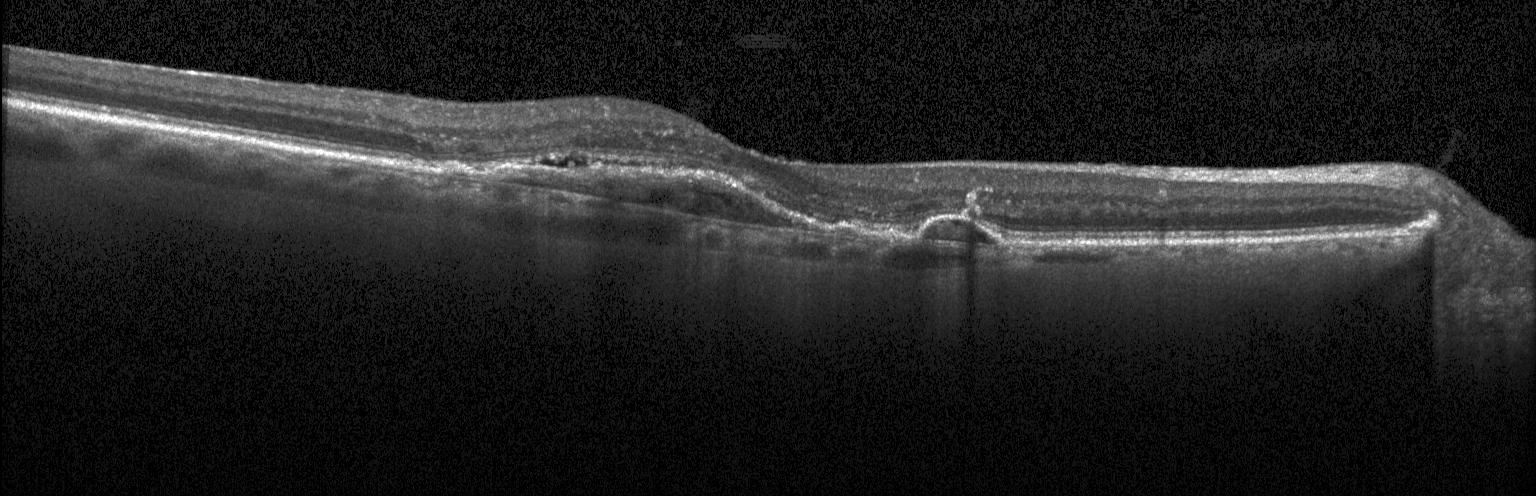

Spectral-domain optical coherence tomography, retinal OCT B-scan, acquired on a Heidelberg Spectralis, fovea-centered
Finding: choroidal neovascularization.